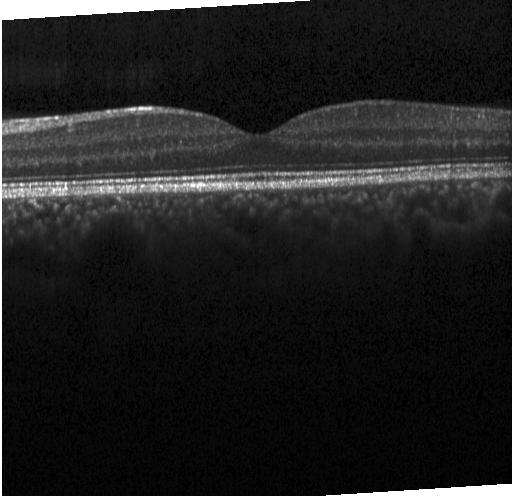 OCT line scan · Heidelberg Spectralis OCT system
This B-scan demonstrates no evidence of CNV, DME, or drusen.